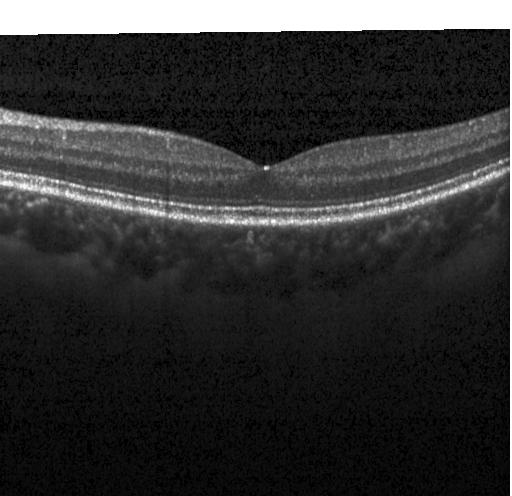

Retinal OCT cross-section
Finding: neither choroidal neovascularization, diabetic macular edema, nor drusen.